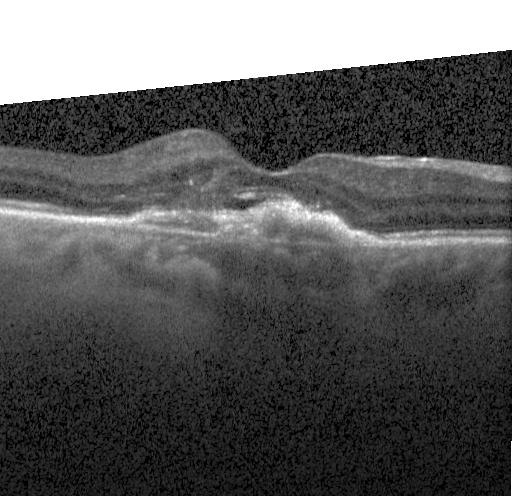 Spectral-domain OCT. Through the macula. Heidelberg Spectralis. Optical coherence tomography B-scan.
Finding: choroidal neovascularization.